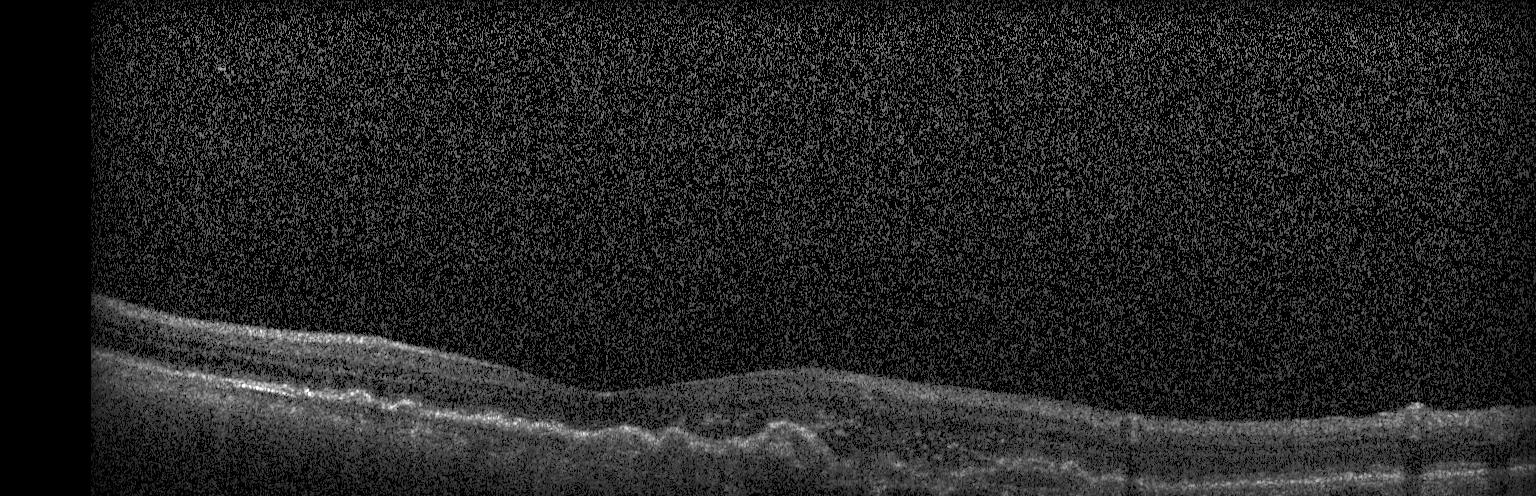
Heidelberg Spectralis · horizontal scan through the fovea · spectral-domain optical coherence tomography · optical coherence tomography B-scan. Assessment: a choroidal neovascular membrane.